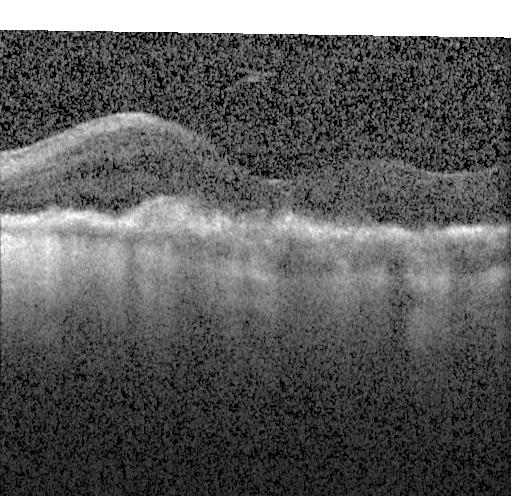
Retinal OCT B-scan — Assessment: choroidal neovascularization.